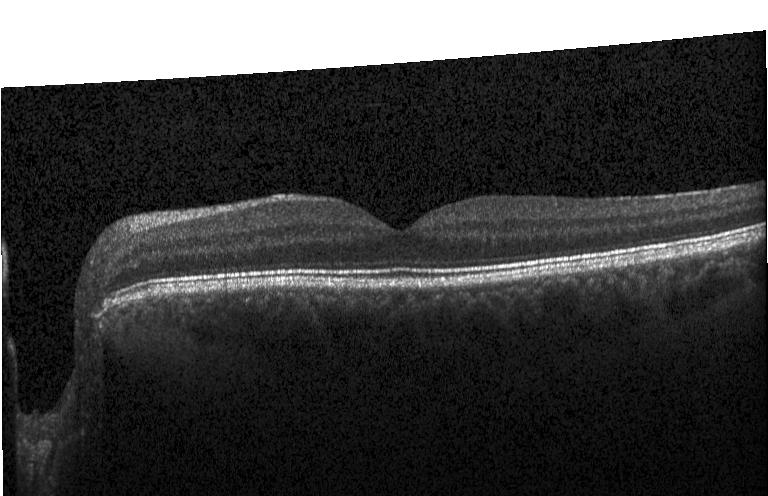

Optical coherence tomography scan, macular scan, Heidelberg Spectralis — The scan shows neither choroidal neovascularization, diabetic macular edema, nor drusen.